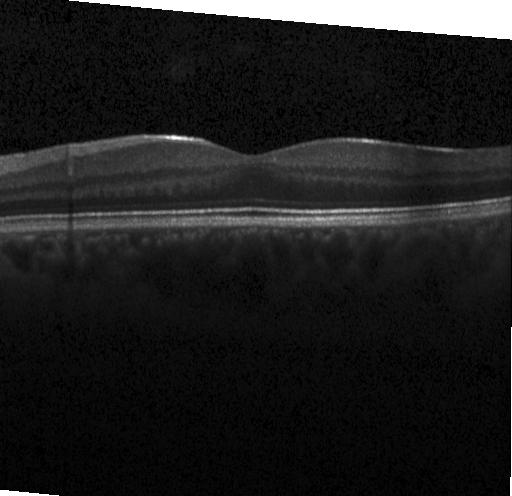

Macular scan · retinal OCT cross-section.
Diagnosis: neither CNV, DME, nor drusen.